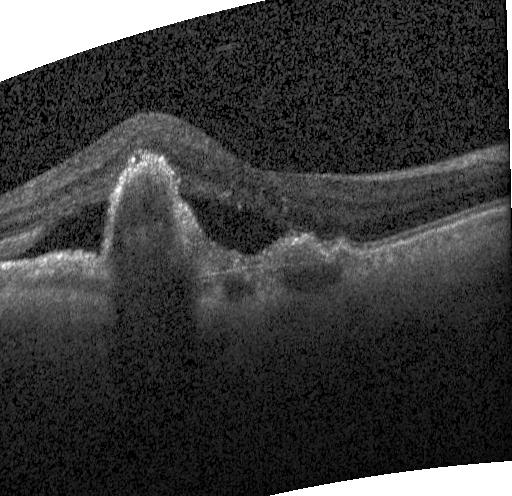 OCT B-scan — The scan shows a choroidal neovascular membrane.